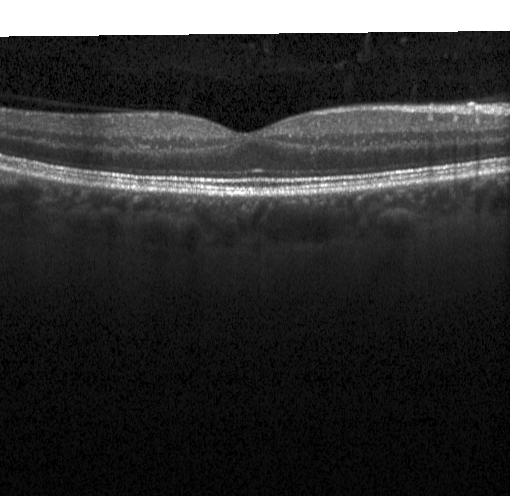
OCT line scan.
Impression: no evidence of choroidal neovascularization, diabetic macular edema, or drusen.